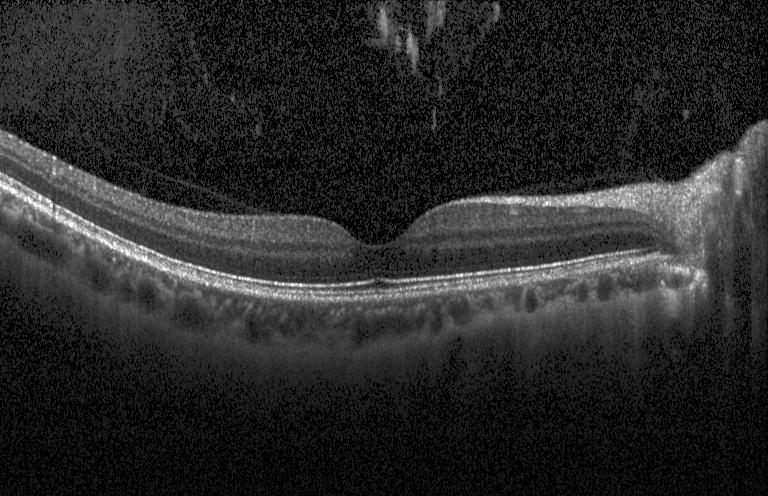
Fovea-centered; instrument: Heidelberg Spectralis; OCT B-scan; spectral-domain OCT. Finding: no choroidal neovascularization, no diabetic macular edema, and no drusen.